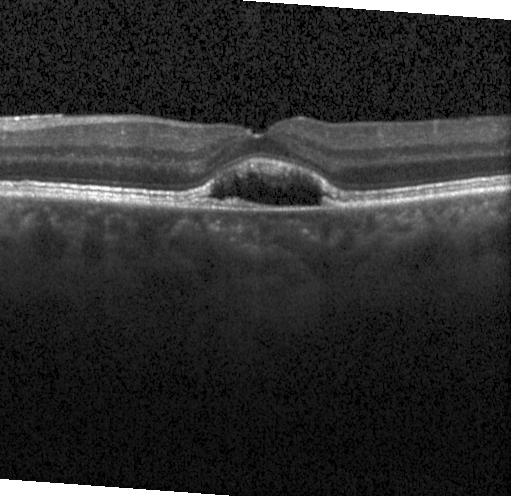 Instrument: Heidelberg Spectralis; retinal OCT cross-section
Macular OCT: a choroidal neovascular membrane.